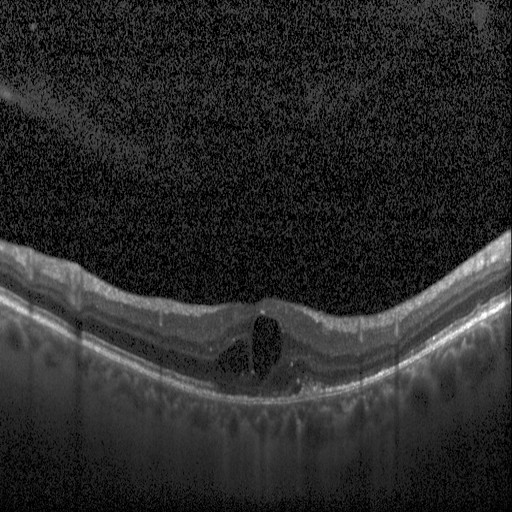

Retinal OCT B-scan — Diabetic macular edema (DME).